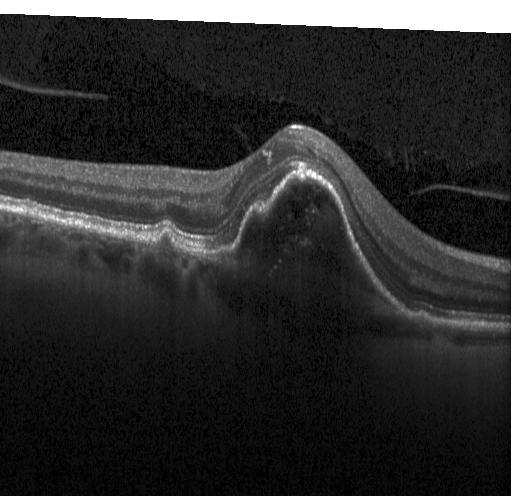
Optical coherence tomography B-scan
Macular OCT: a choroidal neovascular membrane.